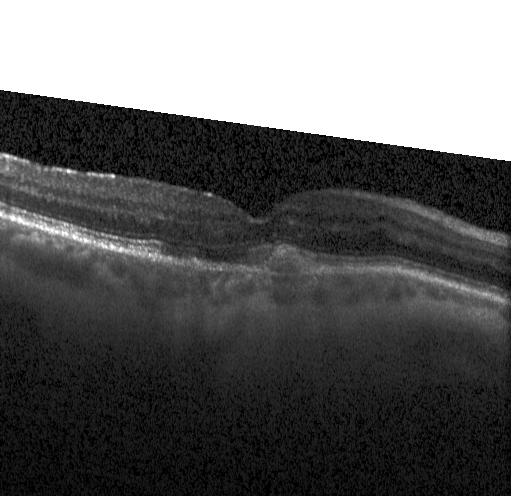
Retinal OCT cross-section showing choroidal neovascularization (CNV).